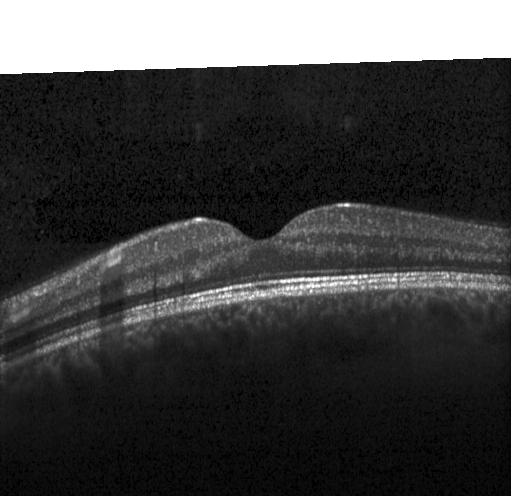 SD-OCT · instrument: Heidelberg Spectralis · optical coherence tomography B-scan
Finding: no choroidal neovascularization, no diabetic macular edema, and no drusen.